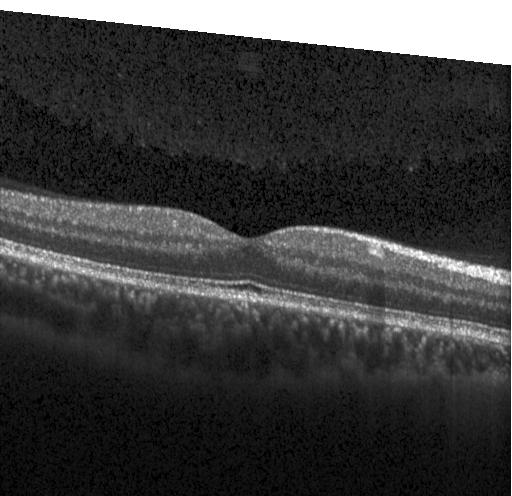

Diagnosis: no CNV, no DME, and no drusen.